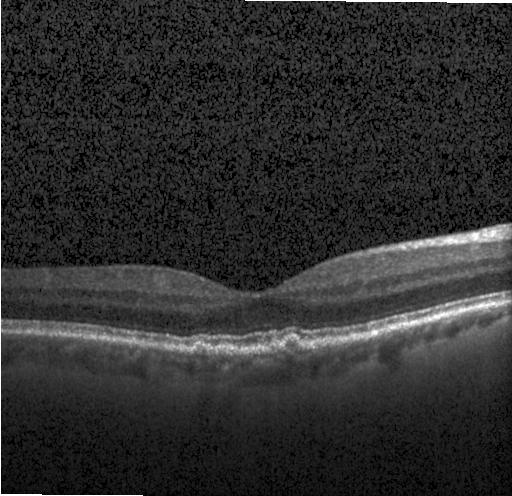 Retinal OCT cross-section showing drusen.